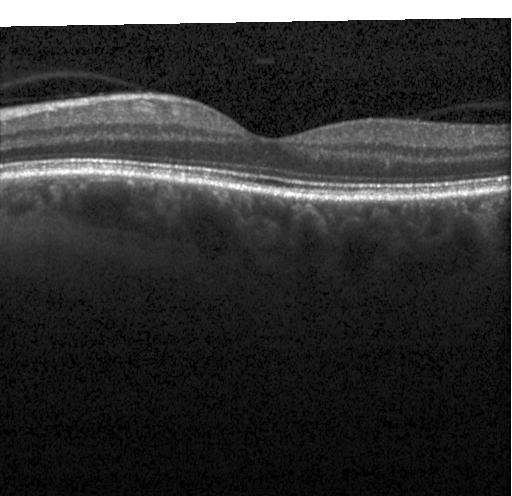 Macular OCT: no choroidal neovascularization, diabetic macular edema, or drusen.